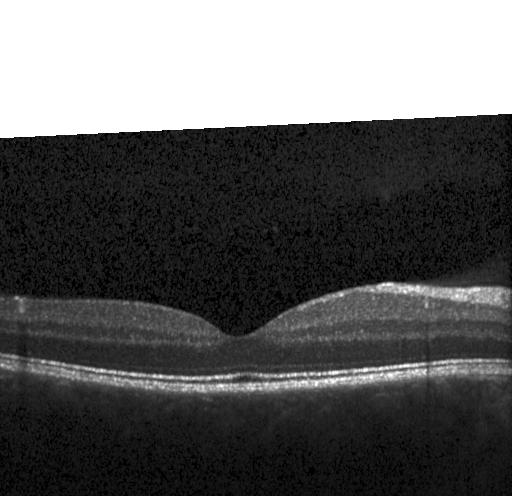 Diagnosis: neither CNV, DME, nor drusen.